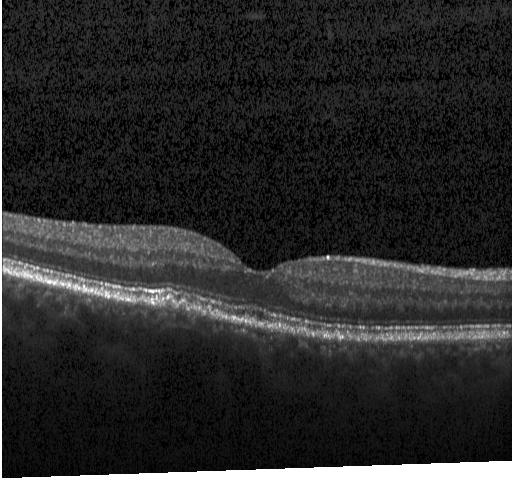

Optical coherence tomography B-scan, horizontal scan through the fovea, acquired on a Heidelberg Spectralis, spectral-domain OCT. Finding: drusen.